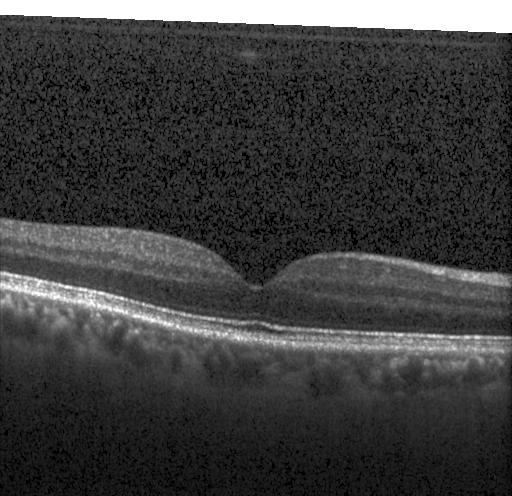 OCT scan showing neither choroidal neovascularization, diabetic macular edema, nor drusen.